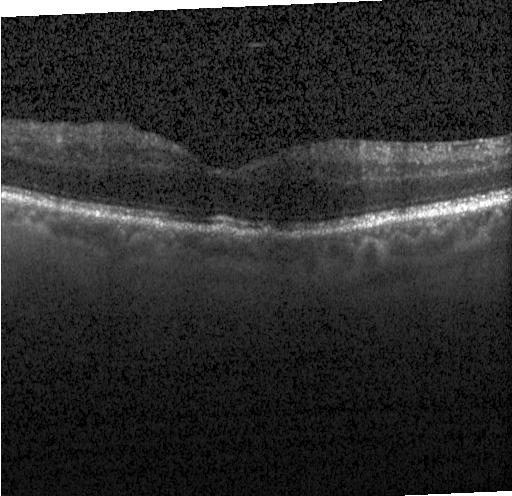
Instrument: Heidelberg Spectralis, spectral-domain optical coherence tomography, through the macula, OCT line scan.
This B-scan demonstrates neither choroidal neovascularization, diabetic macular edema, nor drusen.